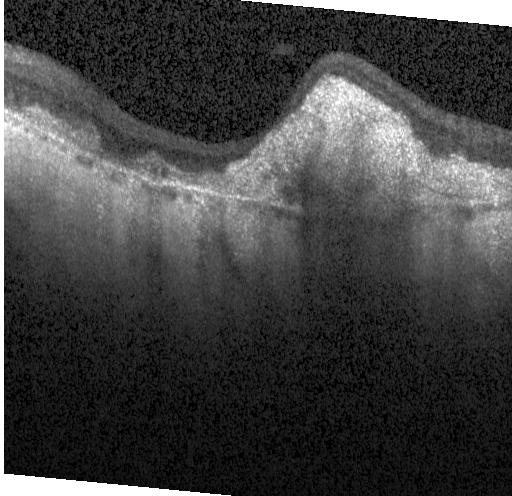
Optical coherence tomography B-scan
Finding: choroidal neovascularization.